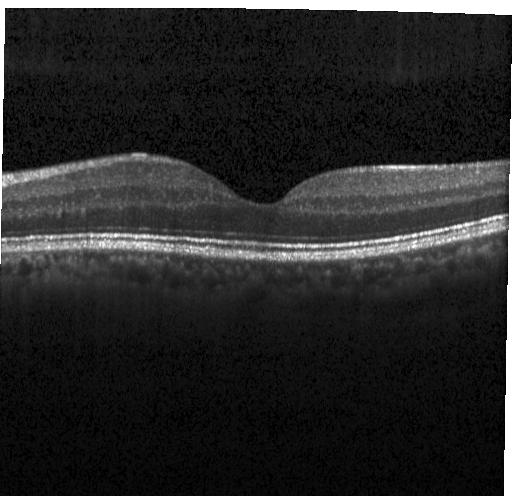

OCT B-scan showing no CNV, no DME, and no drusen.